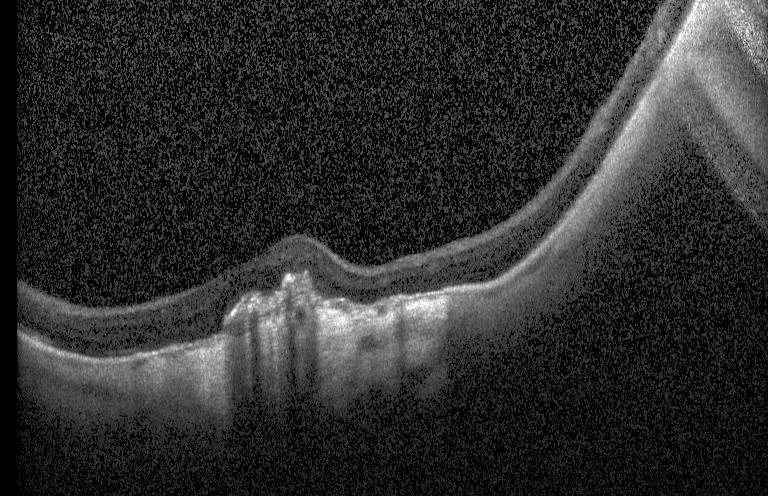 The scan shows a choroidal neovascular membrane.